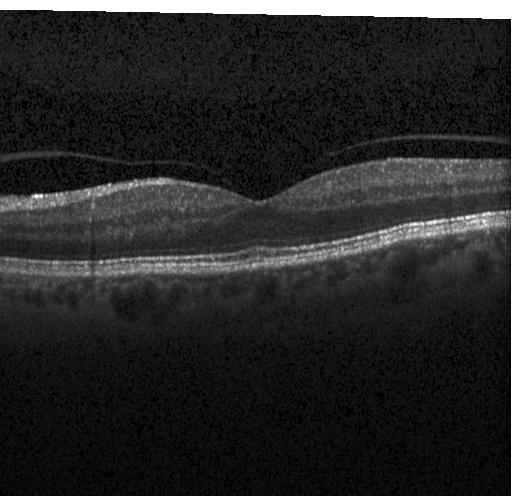 This B-scan demonstrates no choroidal neovascularization, diabetic macular edema, or drusen.